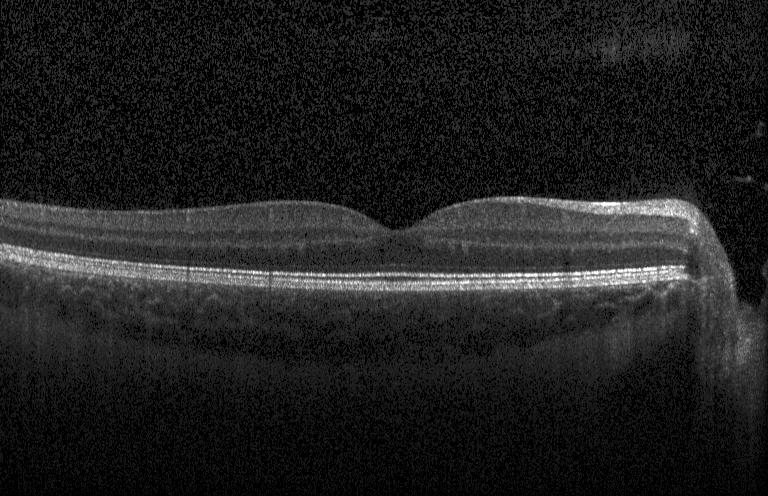 Spectral-domain OCT, OCT B-scan, through the macula, instrument: Heidelberg Spectralis.
Assessment: no CNV, no DME, and no drusen.